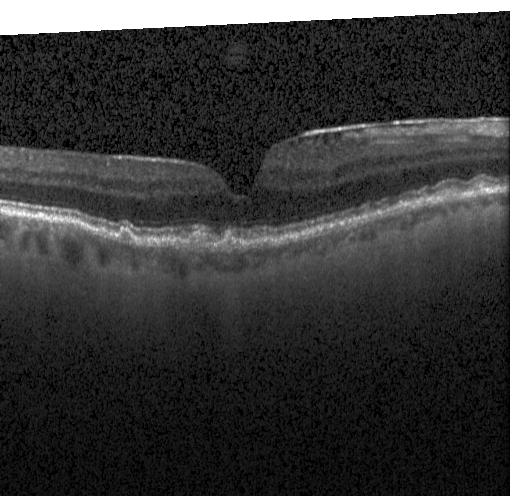
Macular OCT demonstrating drusen.